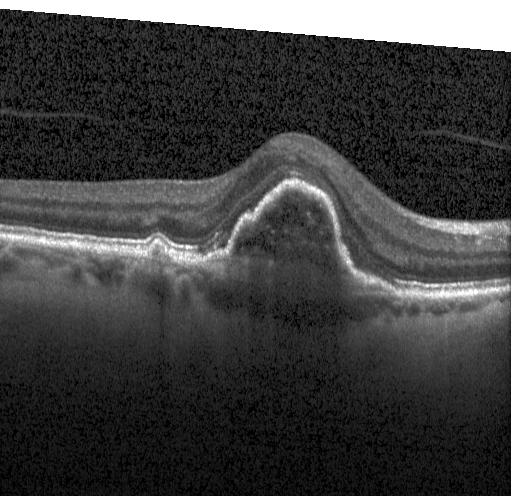
OCT B-scan.
Finding: CNV.